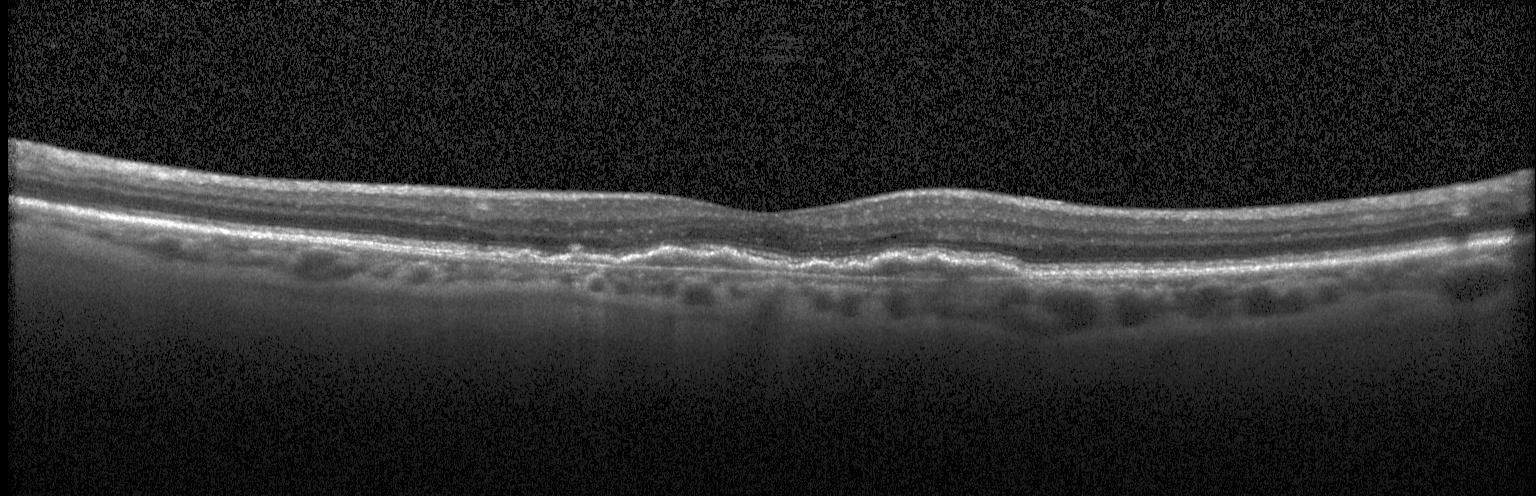
This B-scan demonstrates a choroidal neovascular membrane.